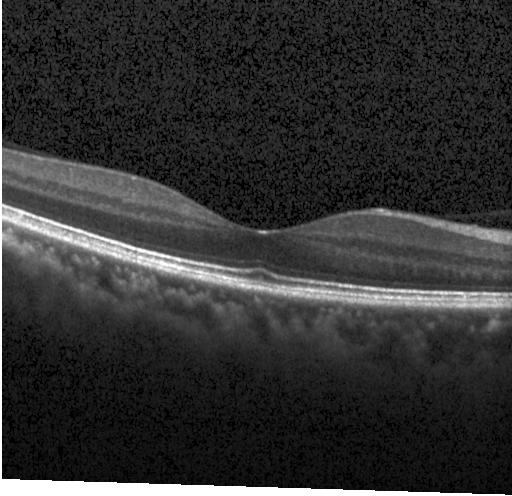 OCT B-scan showing no choroidal neovascularization, diabetic macular edema, or drusen.